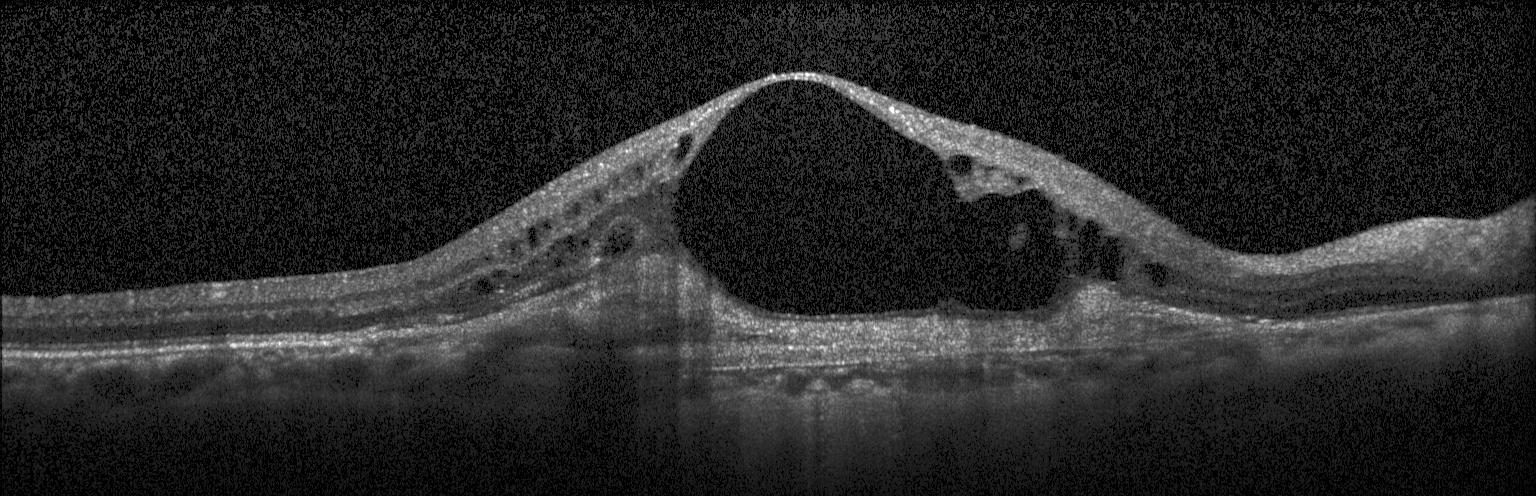 Spectral-domain OCT. Retinal OCT B-scan. Through the macula. Instrument: Heidelberg Spectralis — Diagnosis: a choroidal neovascular membrane.